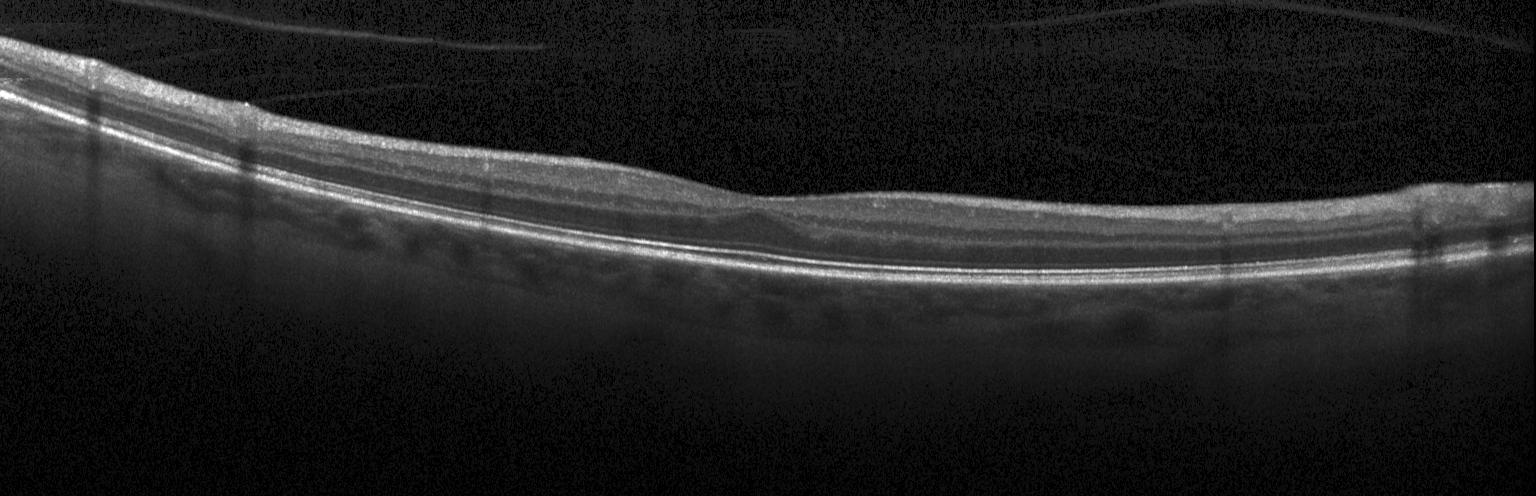
Spectral-domain OCT. Fovea-centered. Optical coherence tomography B-scan. Assessment: no choroidal neovascularization, no diabetic macular edema, and no drusen.